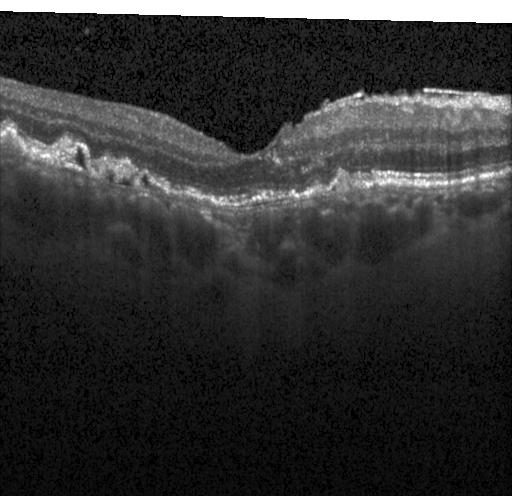

OCT B-scan; Heidelberg Spectralis — Finding: CNV.